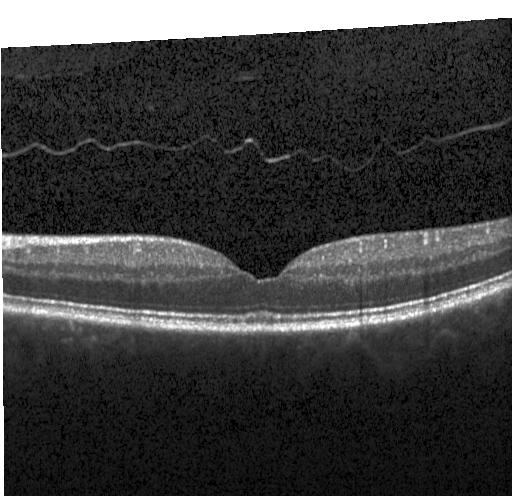

Optical coherence tomography scan.
Finding: no CNV, DME, or drusen.